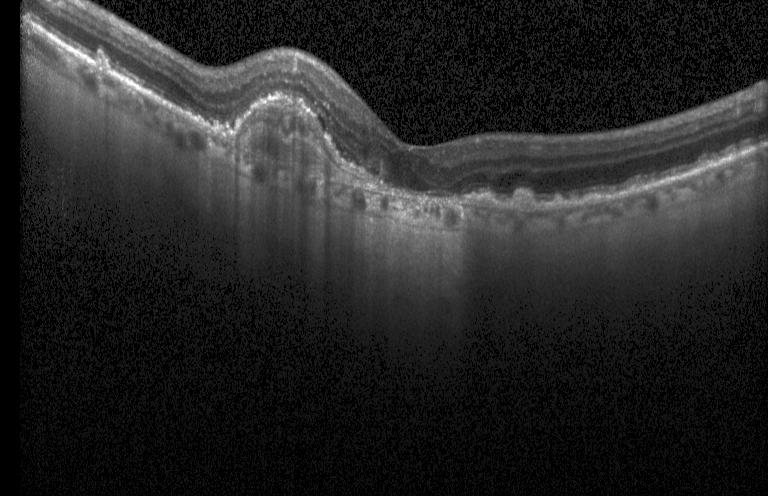

Retinal OCT B-scan. Acquired on a Heidelberg Spectralis. Centered on the fovea.
The scan shows a choroidal neovascular membrane.